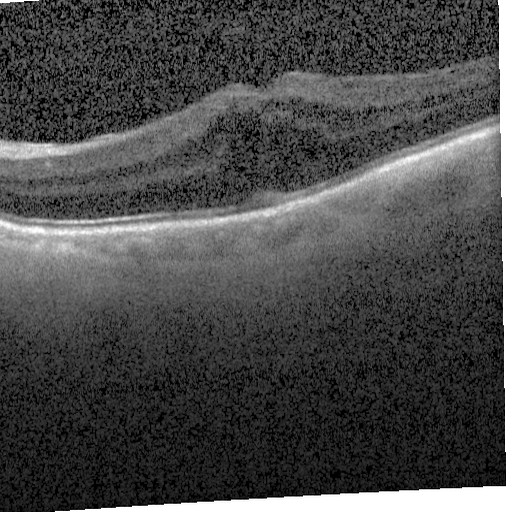
This B-scan demonstrates DME.